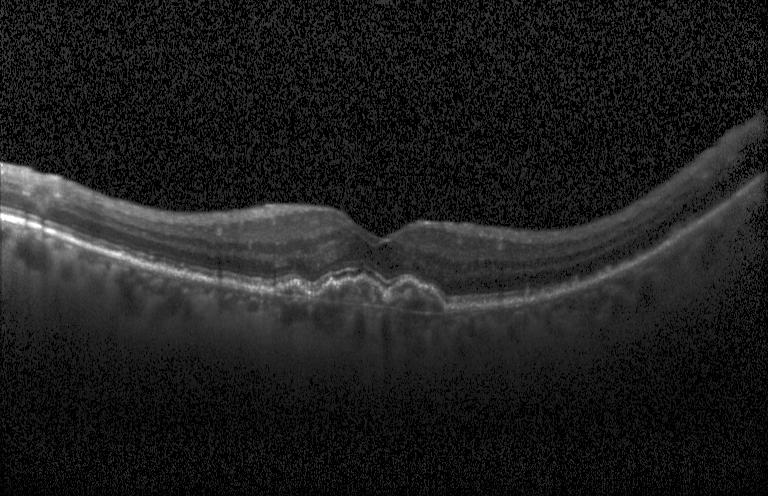
OCT line scan.
Impression: choroidal neovascularization (CNV).